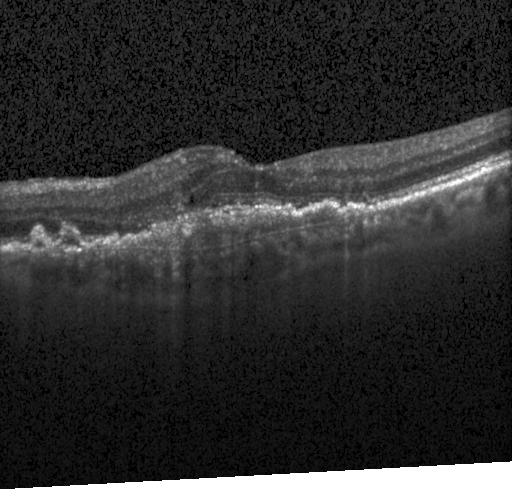
Optical coherence tomography scan — OCT finding: choroidal neovascularization.